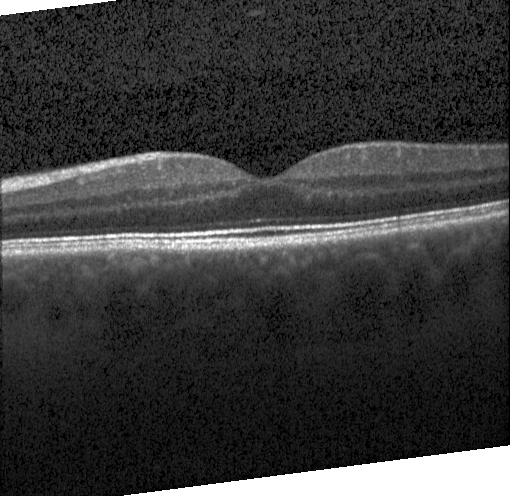

Acquired on a Heidelberg Spectralis, macular scan, retinal OCT B-scan
Dx: no evidence of choroidal neovascularization, diabetic macular edema, or drusen.